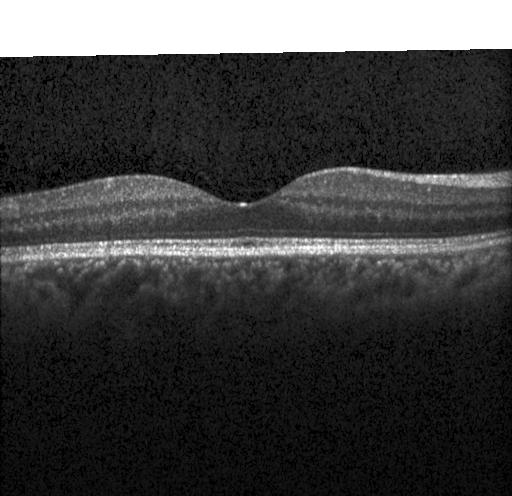

OCT line scan · through the macula · Heidelberg Spectralis. Macular OCT: neither choroidal neovascularization, diabetic macular edema, nor drusen.